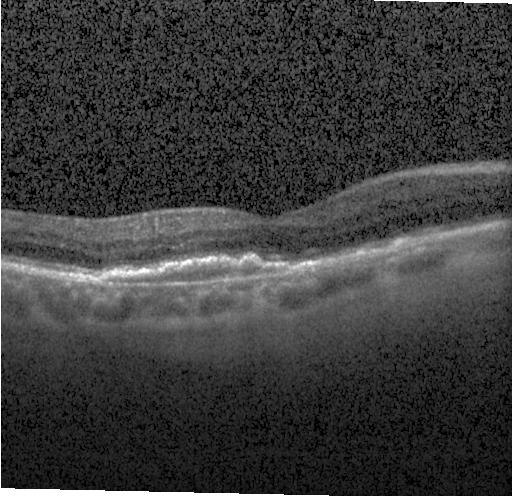 Spectral-domain optical coherence tomography; retinal OCT B-scan; acquired on a Heidelberg Spectralis.
The scan shows a choroidal neovascular membrane.